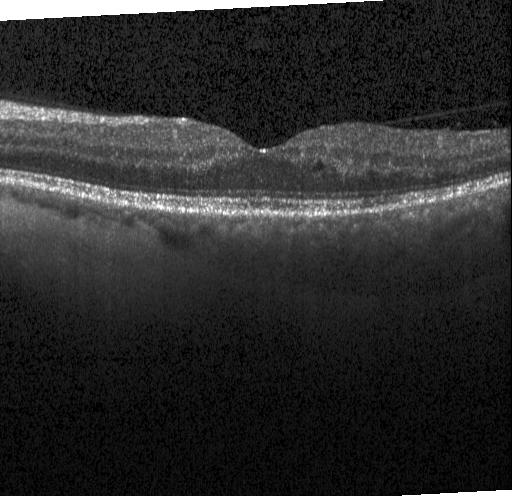

OCT B-scan showing diabetic macular edema (DME).